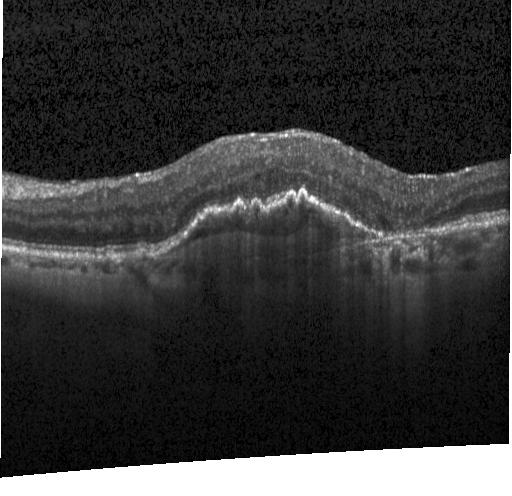

Retinal OCT cross-section showing choroidal neovascularization (CNV).